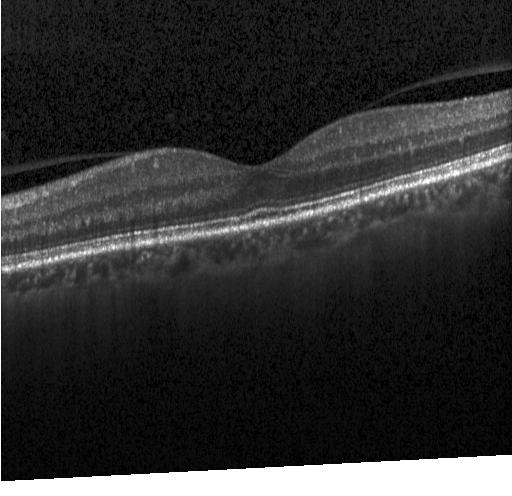
OCT line scan
Macular OCT: no choroidal neovascularization, diabetic macular edema, or drusen.